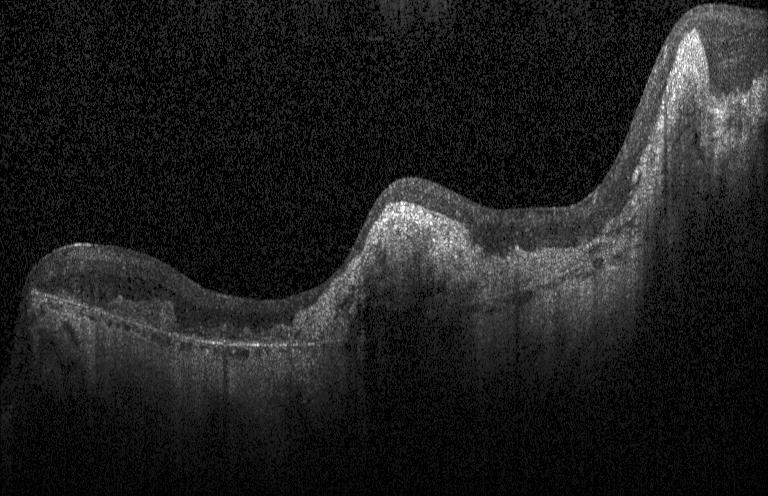 SD-OCT. Optical coherence tomography scan. Acquired on a Heidelberg Spectralis.
Dx: choroidal neovascularization (CNV).